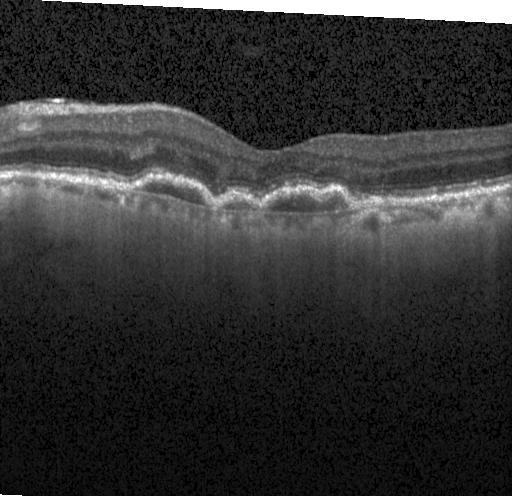 OCT B-scan showing CNV.